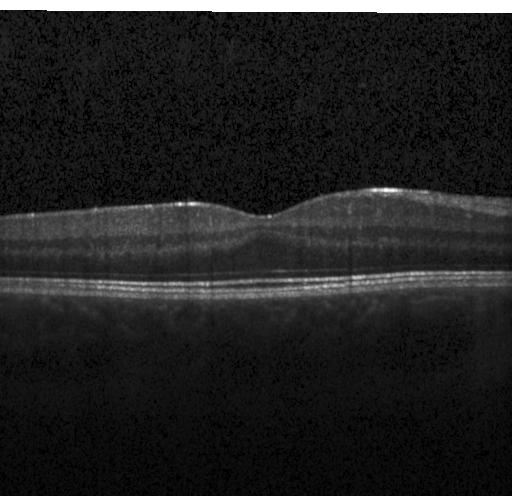 Impression: no evidence of CNV, DME, or drusen.